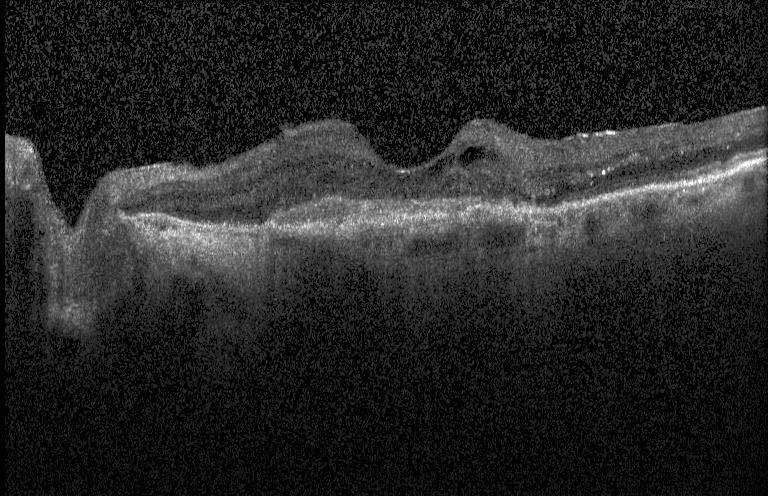

OCT line scan.
Impression: a choroidal neovascular membrane.